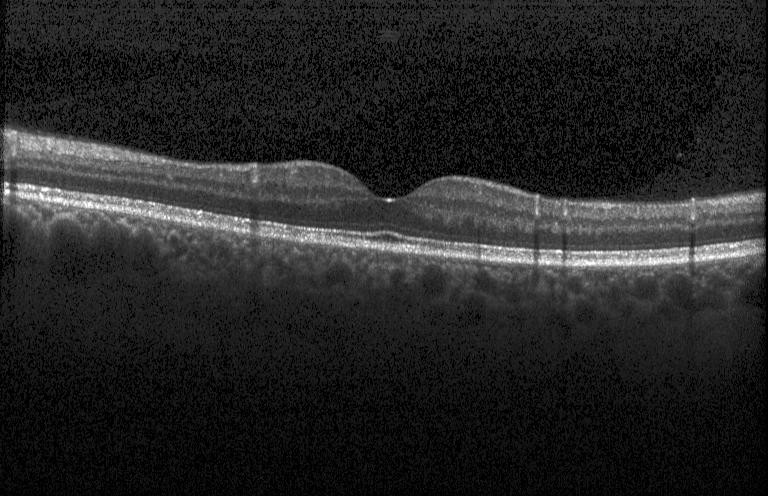
Macular scan. OCT B-scan. Dx: no evidence of choroidal neovascularization, diabetic macular edema, or drusen.